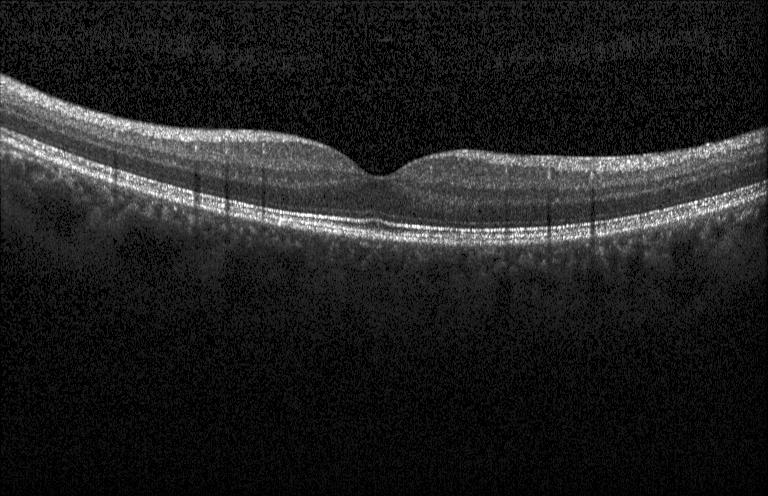
OCT B-scan, instrument: Heidelberg Spectralis. Impression: no choroidal neovascularization, diabetic macular edema, or drusen.